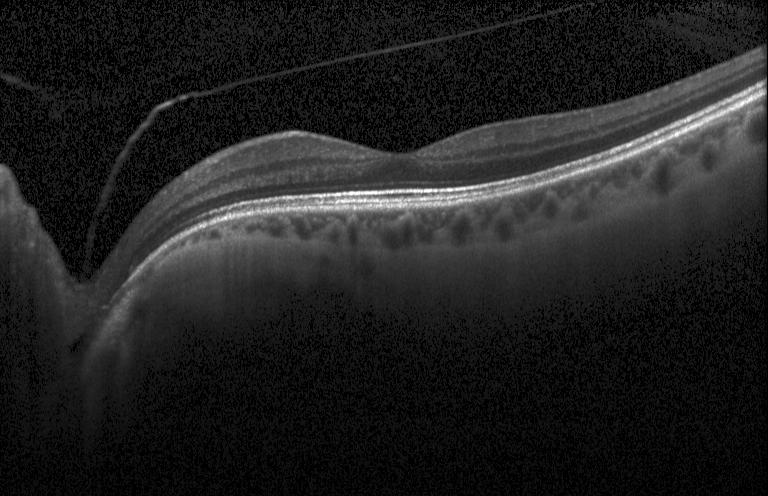
OCT B-scan. Macular OCT: no evidence of CNV, DME, or drusen.